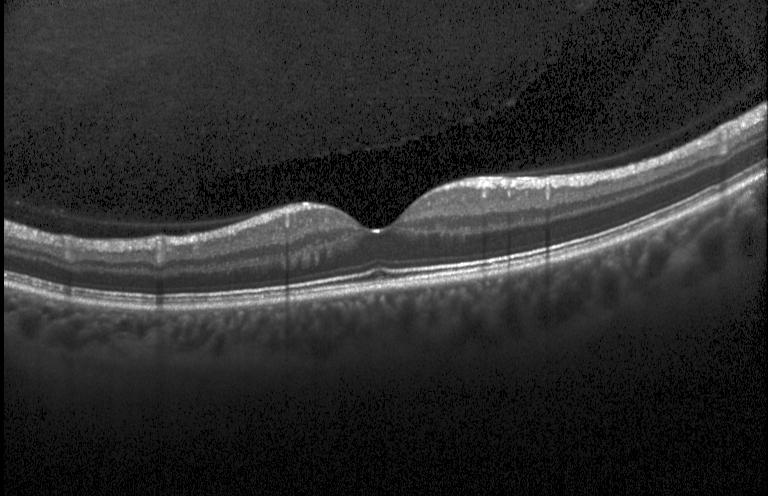 Retinal OCT cross-section, fovea-centered — Diagnosis: no CNV, DME, or drusen.